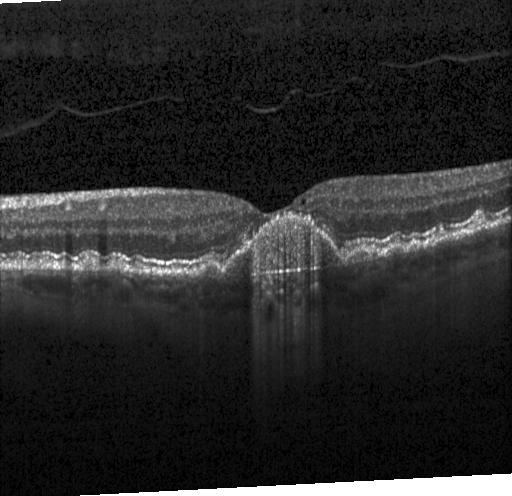

Acquired on a Heidelberg Spectralis. Optical coherence tomography B-scan. Centered on the fovea
This B-scan demonstrates choroidal neovascularization (CNV).